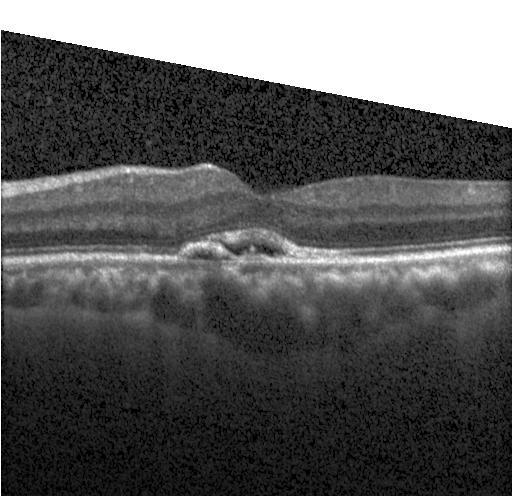

Diagnosis: CNV.